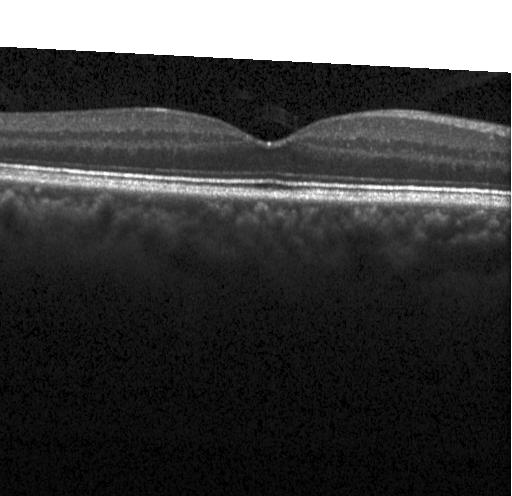

The scan shows neither choroidal neovascularization, diabetic macular edema, nor drusen.